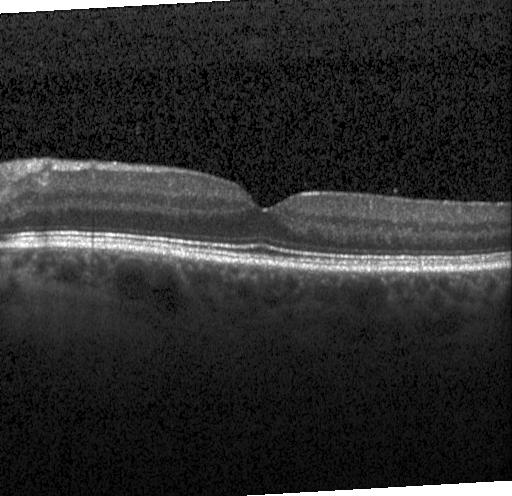 Optical coherence tomography B-scan, through the macula — Dx: no choroidal neovascularization, diabetic macular edema, or drusen.